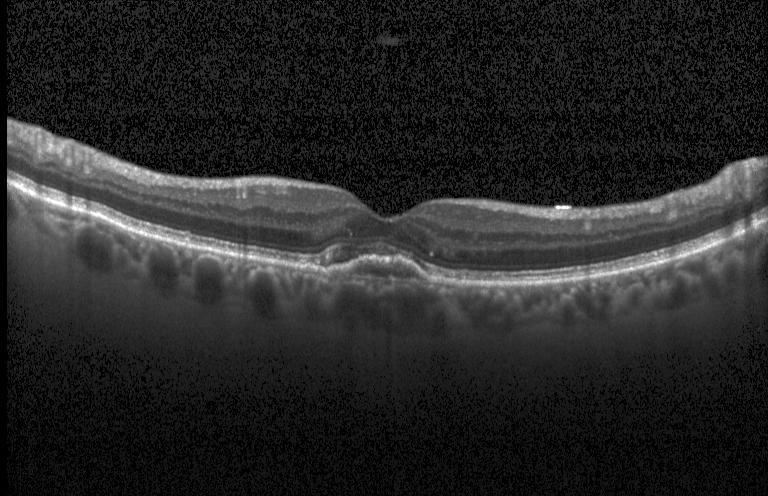 Instrument: Heidelberg Spectralis; OCT B-scan; through the macula; SD-OCT. This B-scan demonstrates CNV.